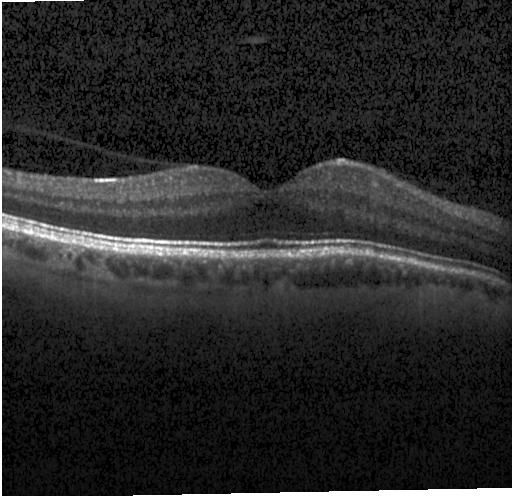
OCT line scan; spectral-domain optical coherence tomography — No evidence of choroidal neovascularization, diabetic macular edema, or drusen.